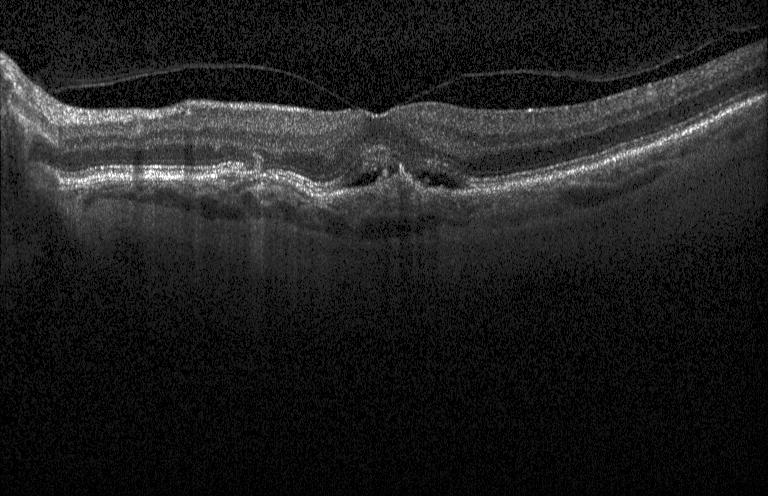

Optical coherence tomography scan, through the macula. Impression: a choroidal neovascular membrane.